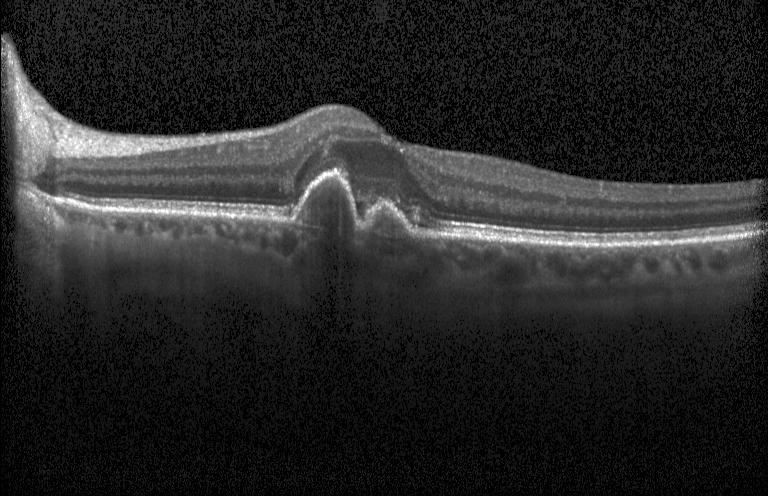
OCT finding: choroidal neovascularization.